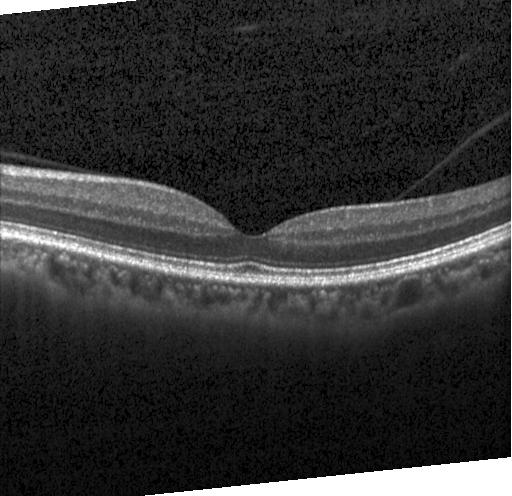

Retinal OCT cross-section. Dx: neither CNV, DME, nor drusen.